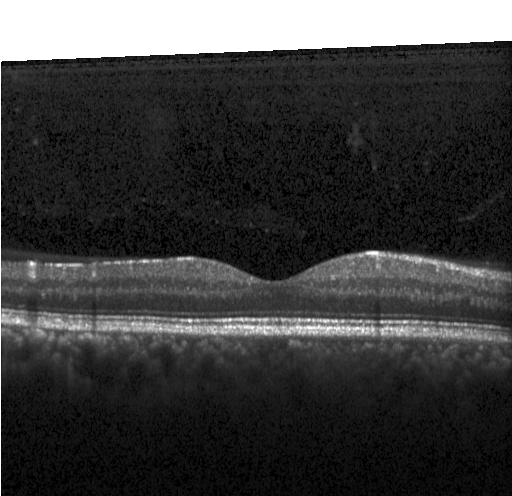

Impression: neither choroidal neovascularization, diabetic macular edema, nor drusen.